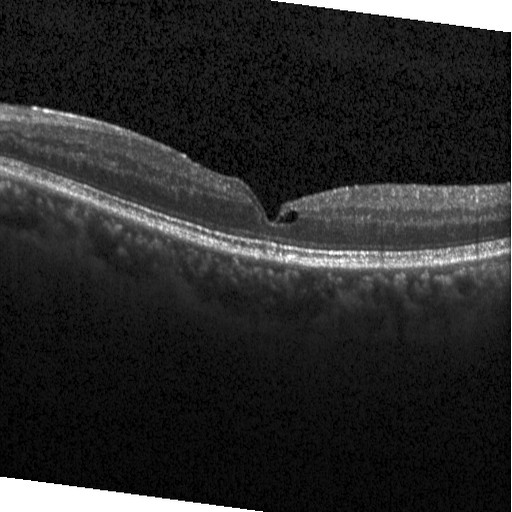 Impression: diabetic macular edema.